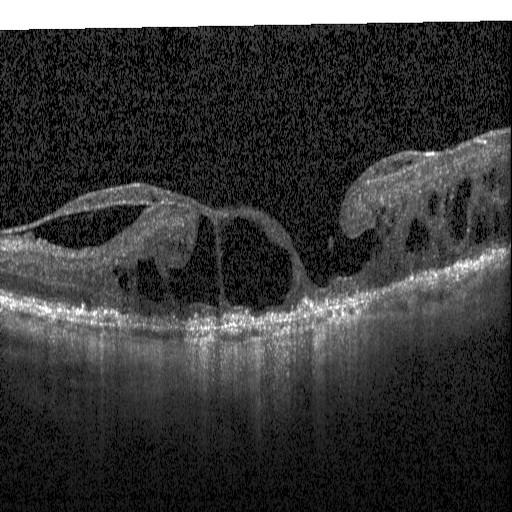 OCT B-scan, spectral-domain OCT, acquired on a Heidelberg Spectralis — Diagnosis: diabetic macular edema (DME).